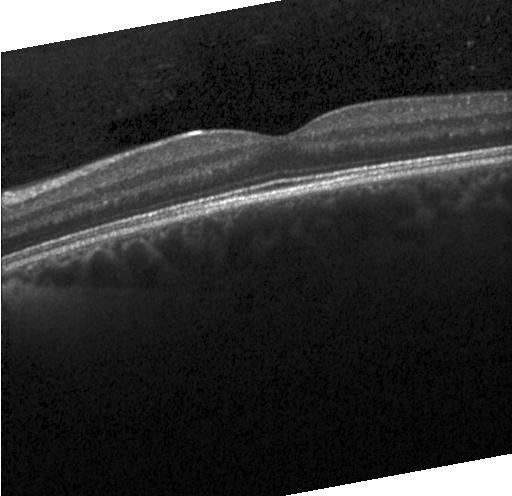
OCT finding: no CNV, DME, or drusen.